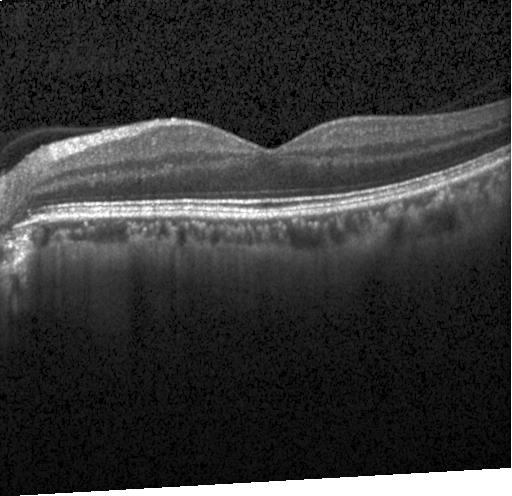 SD-OCT, OCT line scan. The scan shows no evidence of choroidal neovascularization, diabetic macular edema, or drusen.